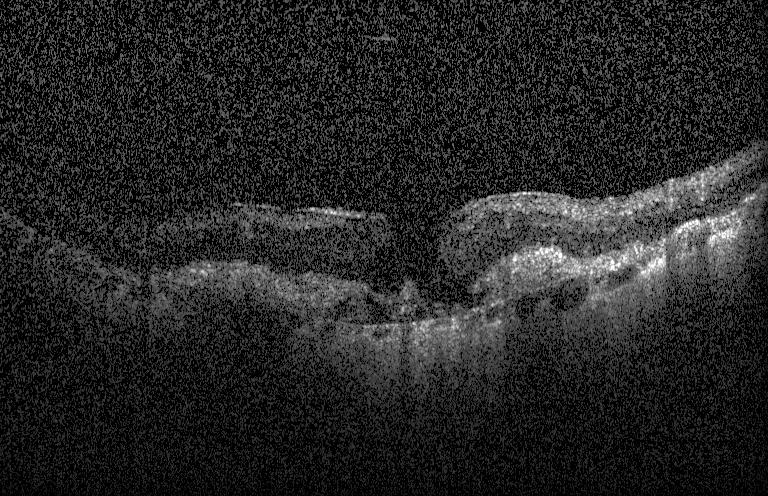

Centered on the fovea; retinal OCT B-scan
Diagnosis: choroidal neovascularization (CNV).